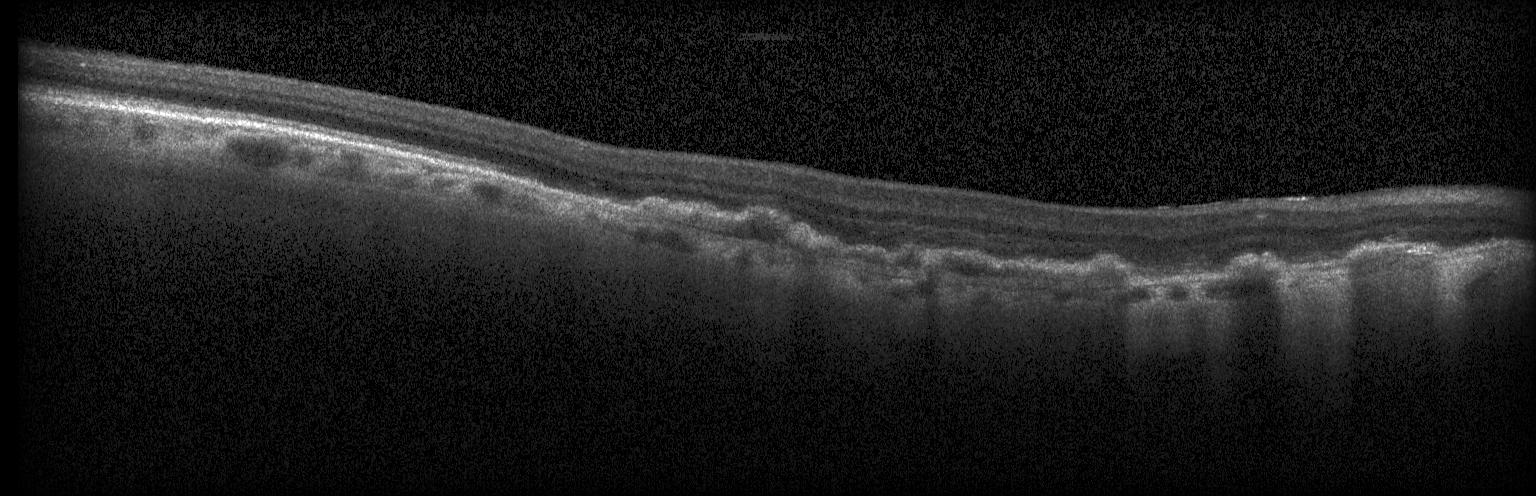 Finding: a choroidal neovascular membrane.